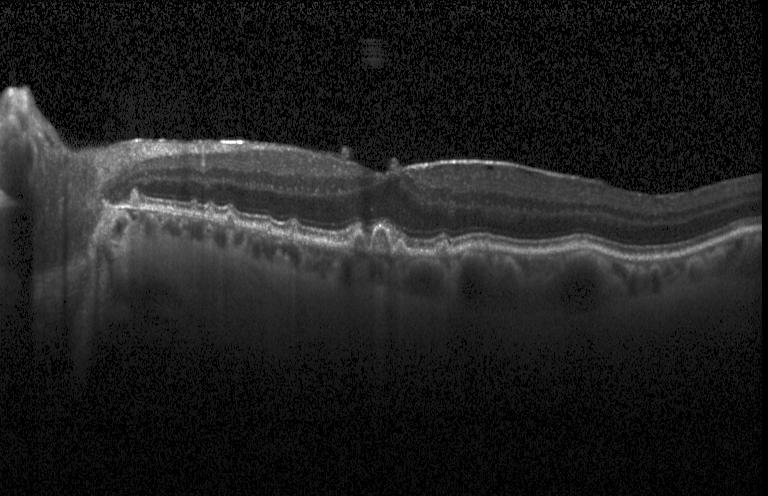 Finding: sub-RPE drusenoid deposits.